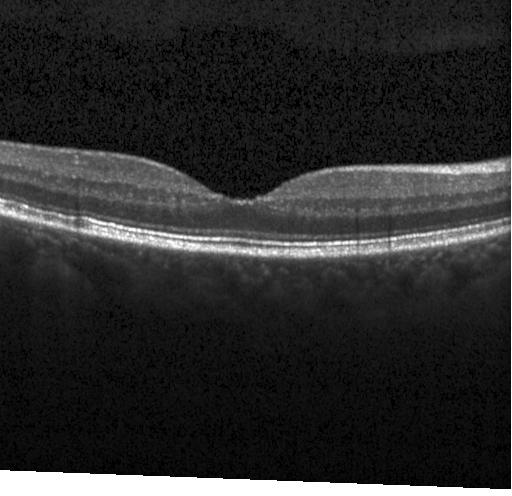

Macular OCT demonstrating no choroidal neovascularization, diabetic macular edema, or drusen.